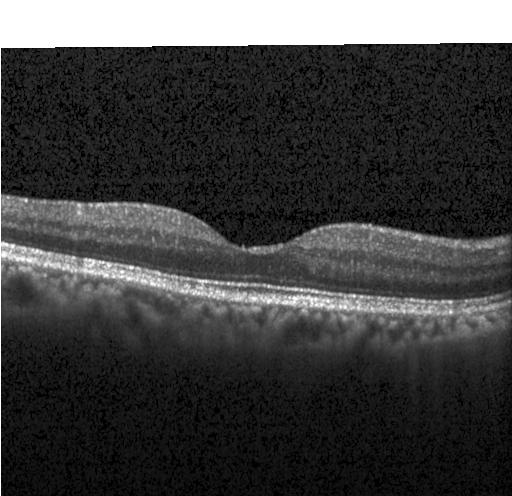

Instrument: Heidelberg Spectralis · retinal OCT B-scan · macular scan — Impression: no CNV, no DME, and no drusen.